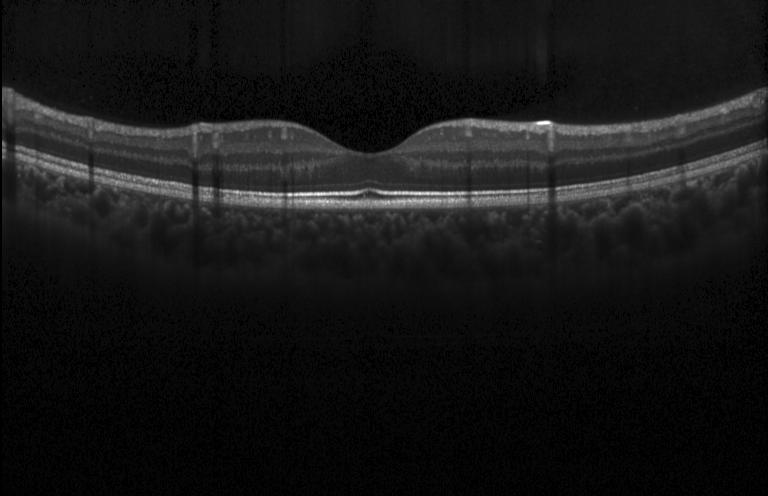

Retinal OCT B-scan — No choroidal neovascularization, no diabetic macular edema, and no drusen.